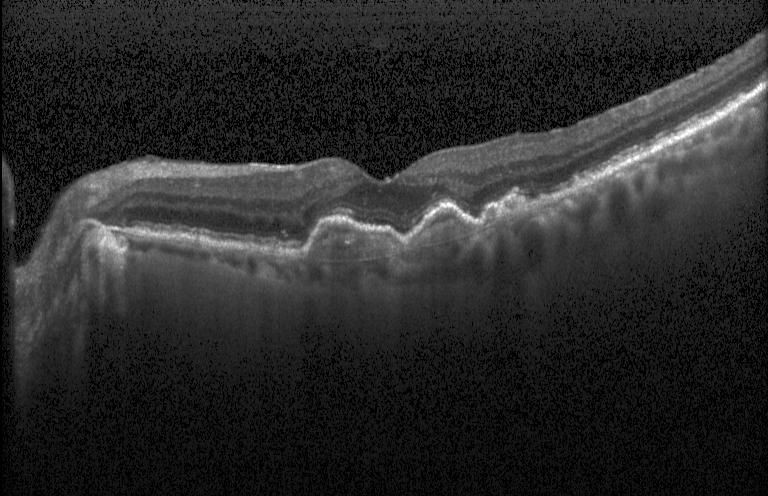 OCT scan showing CNV.